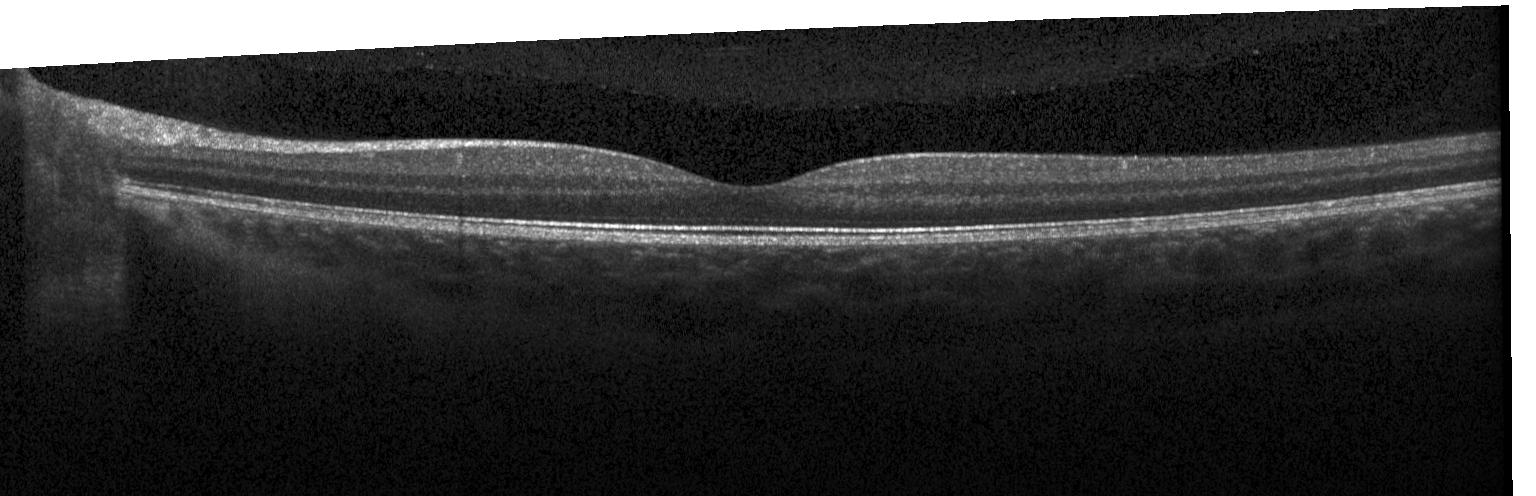 Retinal OCT cross-section. Centered on the fovea. SD-OCT.
Diagnosis: no choroidal neovascularization, diabetic macular edema, or drusen.